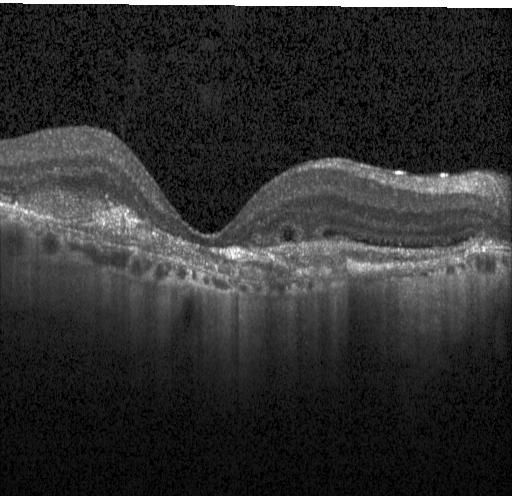 OCT line scan. SD-OCT. Acquired on a Heidelberg Spectralis.
OCT finding: CNV.